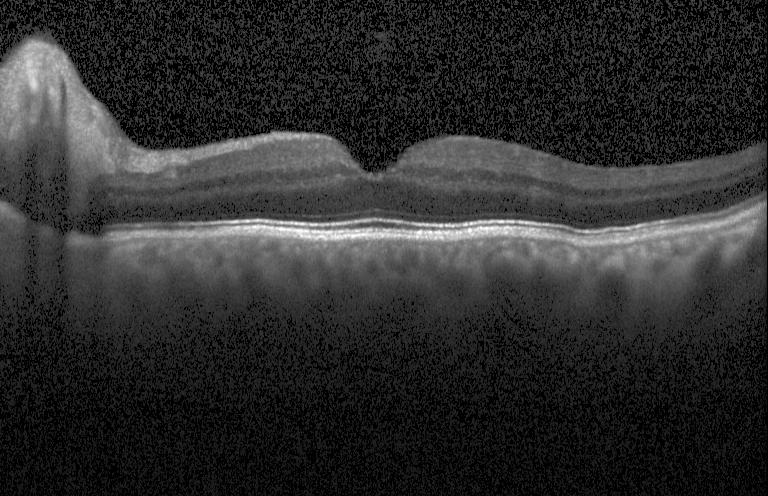 Heidelberg Spectralis; horizontal scan through the fovea; OCT line scan.
No choroidal neovascularization, diabetic macular edema, or drusen.